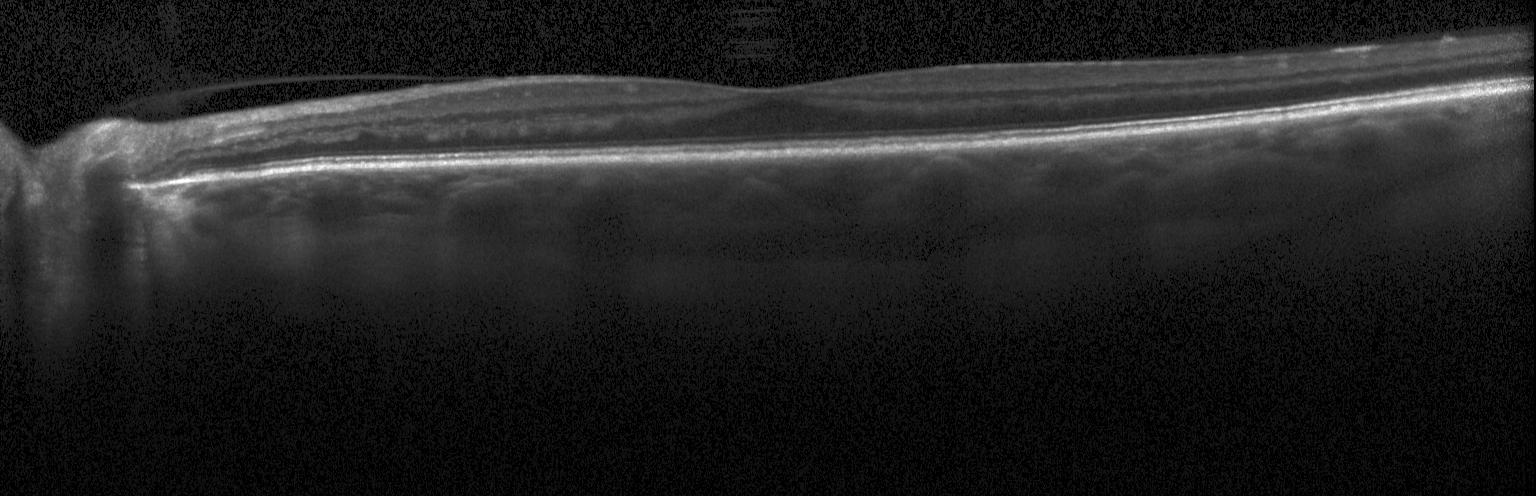

OCT scan showing no evidence of choroidal neovascularization, diabetic macular edema, or drusen.